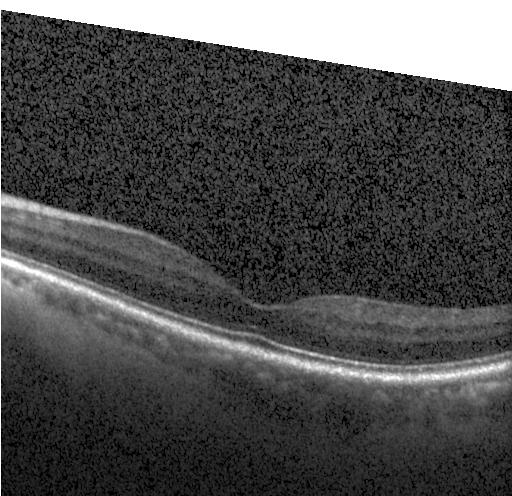

The scan shows no choroidal neovascularization, no diabetic macular edema, and no drusen.